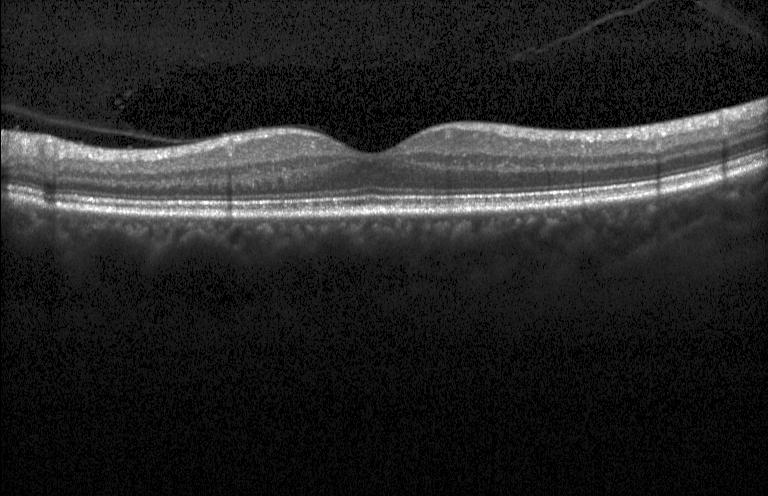 SD-OCT, fovea-centered, Heidelberg Spectralis, OCT line scan.
OCT finding: no choroidal neovascularization, no diabetic macular edema, and no drusen.